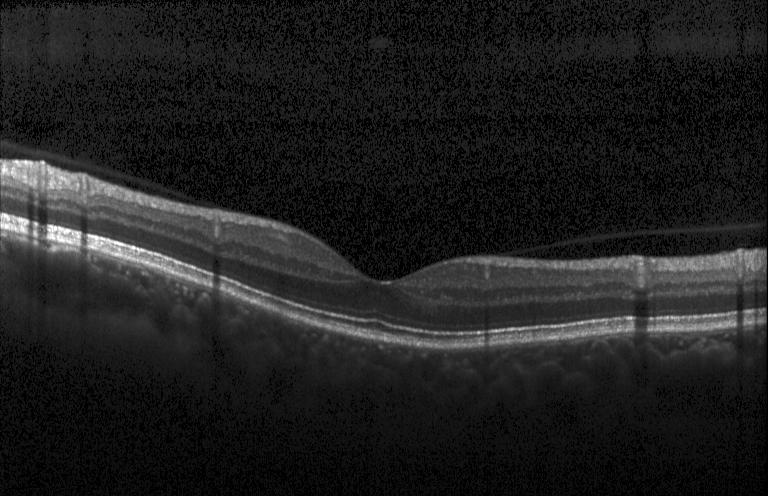 Optical coherence tomography B-scan — Assessment: no CNV, DME, or drusen.